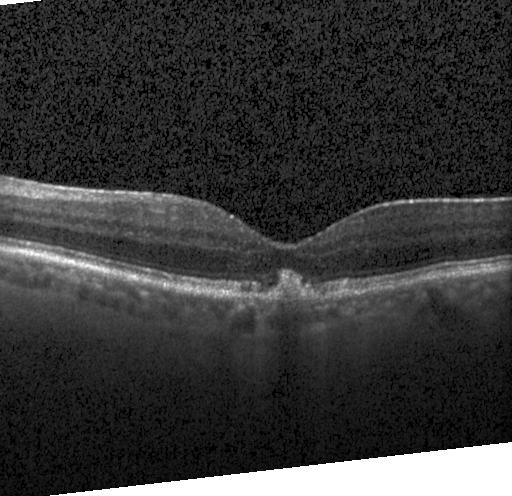

Macular OCT demonstrating a choroidal neovascular membrane.